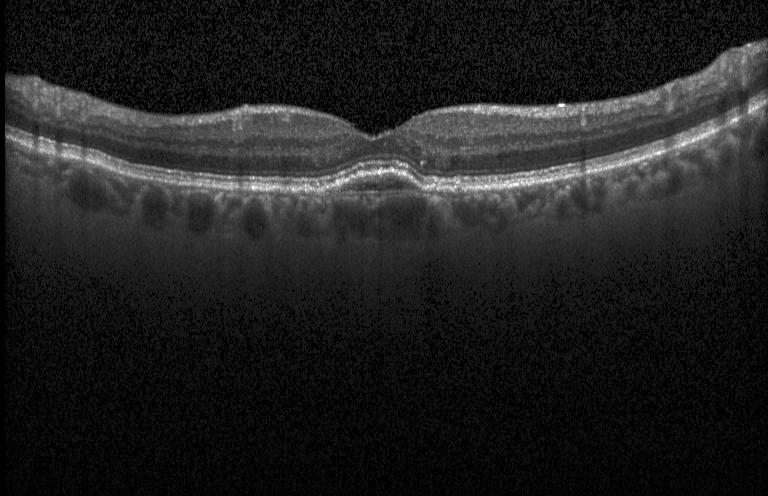

Spectral-domain OCT, retinal OCT B-scan — This B-scan demonstrates a choroidal neovascular membrane.